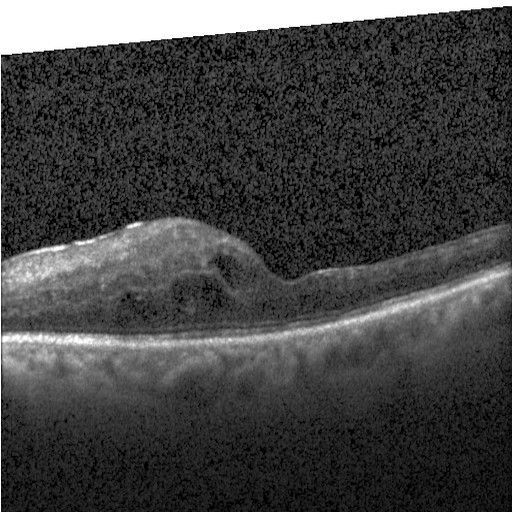

Assessment: DME.